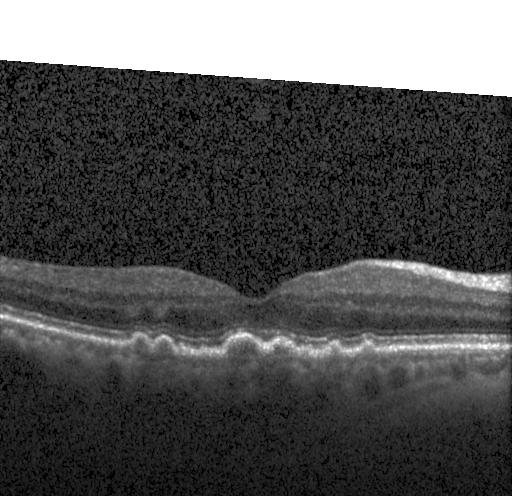 Instrument: Heidelberg Spectralis. Horizontal scan through the fovea. Spectral-domain OCT. Optical coherence tomography B-scan
Finding: multiple drusen.